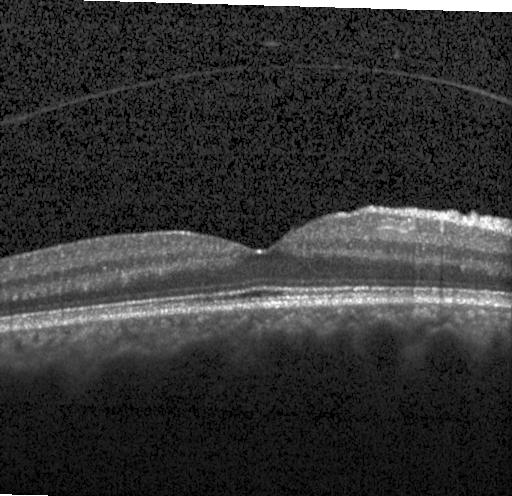 Optical coherence tomography B-scan · through the macula — This B-scan demonstrates no choroidal neovascularization, no diabetic macular edema, and no drusen.